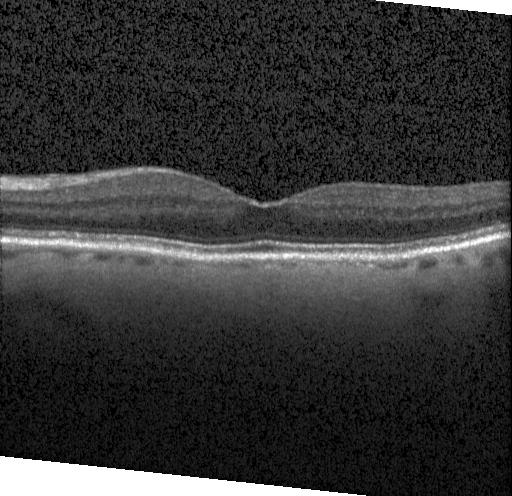
Spectral-domain OCT, retinal OCT B-scan. Macular OCT: no choroidal neovascularization, no diabetic macular edema, and no drusen.